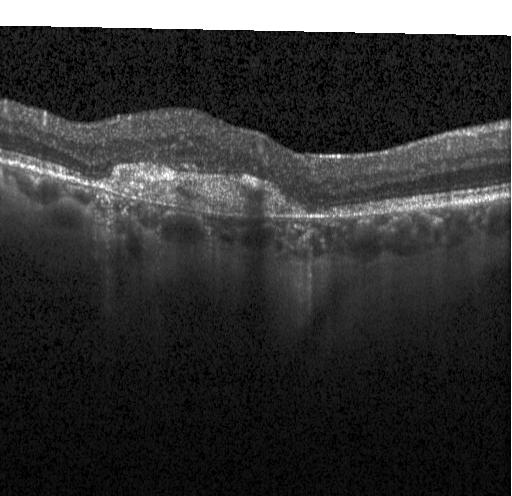
Optical coherence tomography B-scan — OCT finding: CNV.